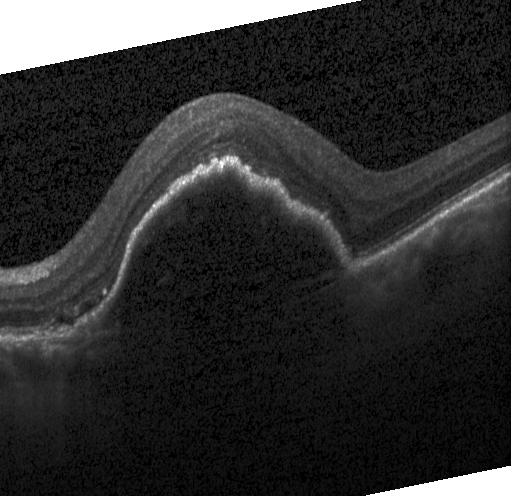 Spectral-domain OCT, retinal OCT B-scan
Macular OCT: a choroidal neovascular membrane.